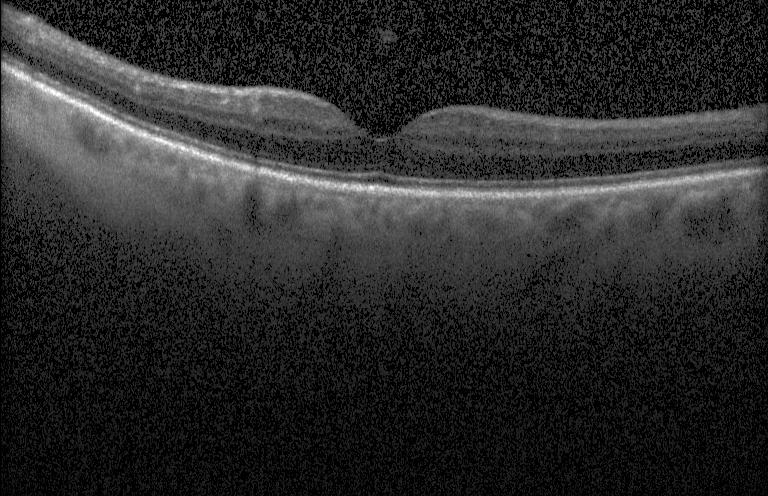

OCT line scan — Impression: no CNV, no DME, and no drusen.